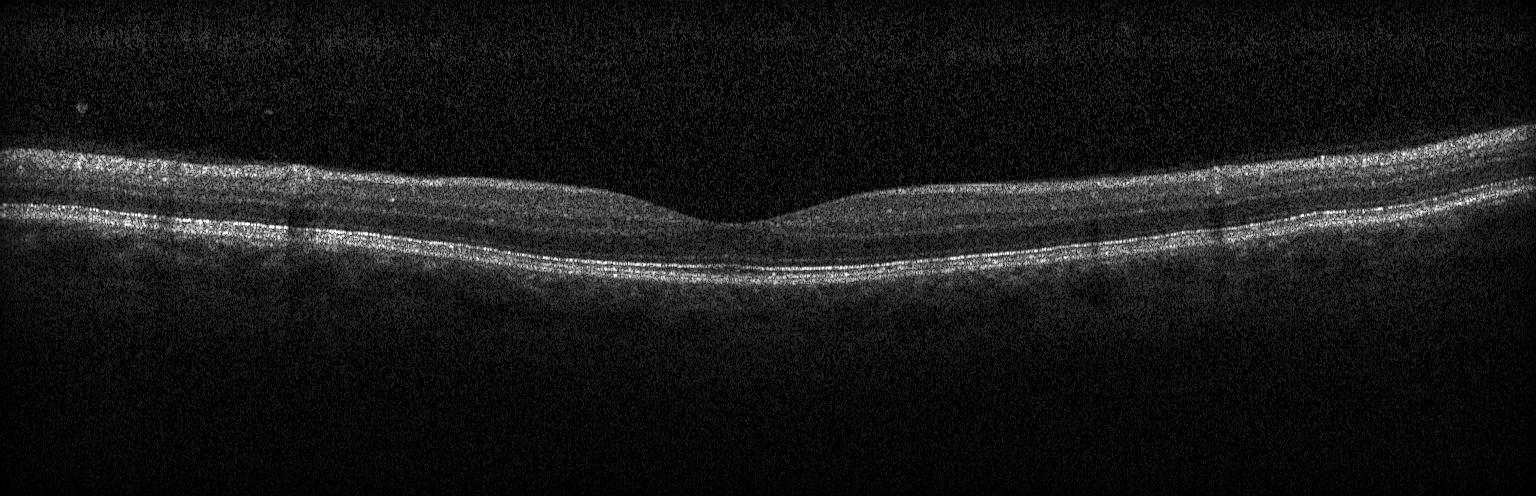

Retinal OCT cross-section.
Impression: no evidence of choroidal neovascularization, diabetic macular edema, or drusen.